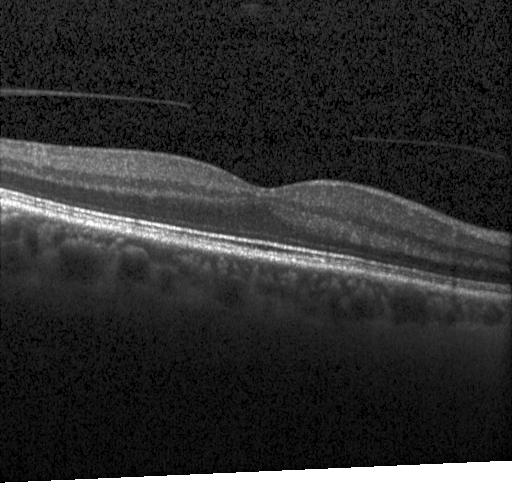 Impression: no CNV, no DME, and no drusen.